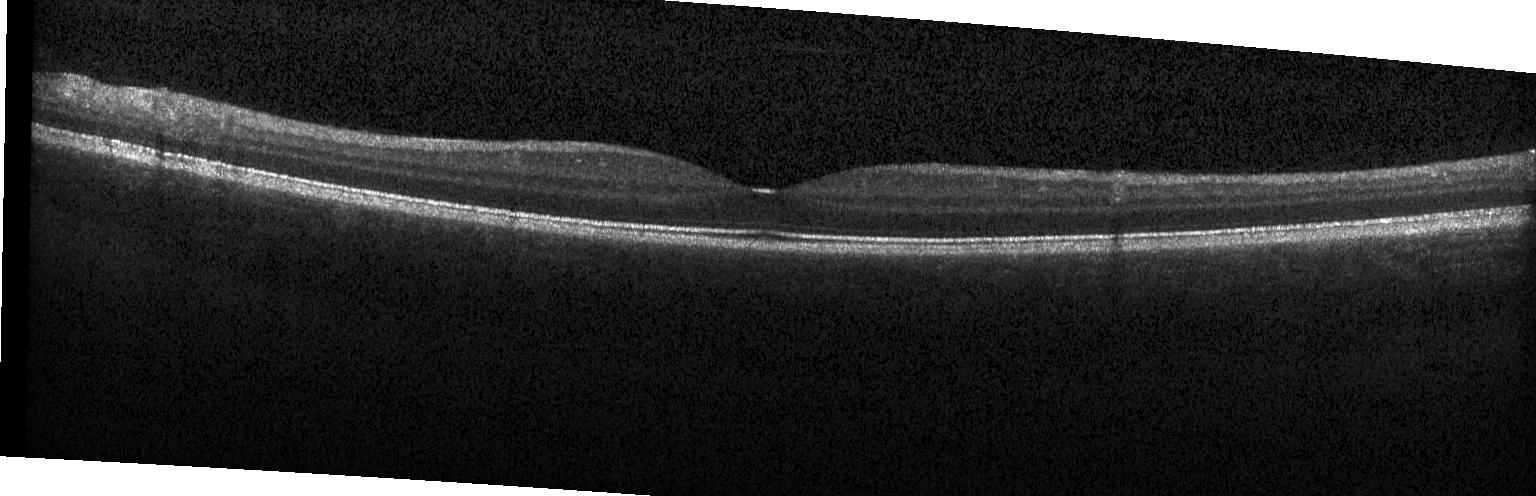 Macular OCT: no CNV, DME, or drusen.